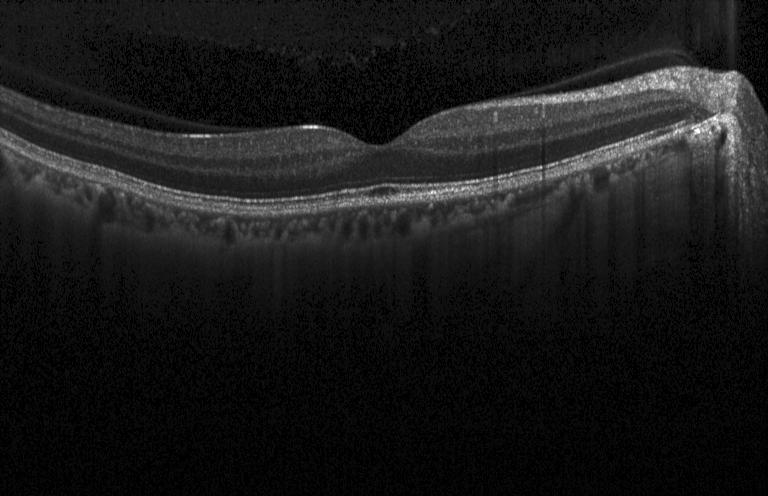
Heidelberg Spectralis · retinal OCT cross-section · spectral-domain optical coherence tomography
Impression: no evidence of choroidal neovascularization, diabetic macular edema, or drusen.